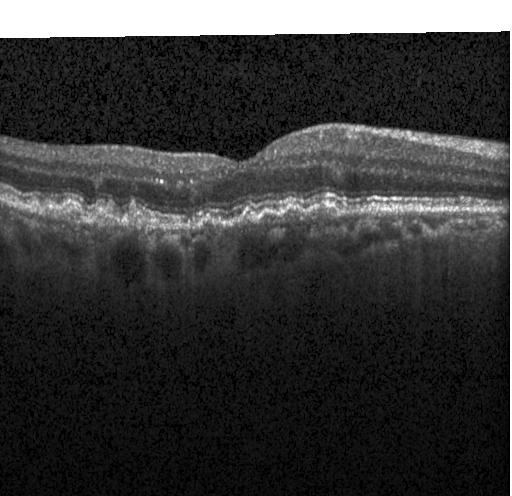
OCT line scan. Impression: sub-RPE drusenoid deposits.